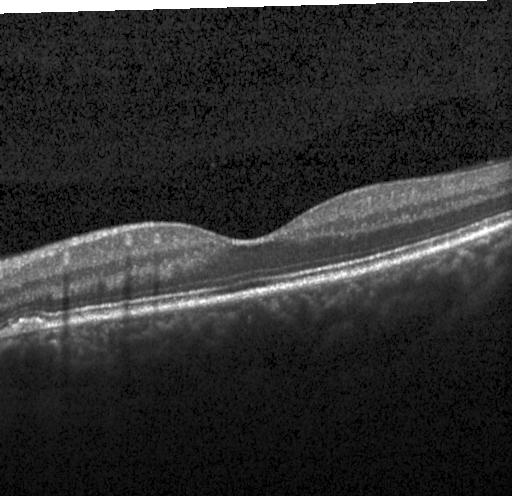
OCT B-scan — Finding: drusen.